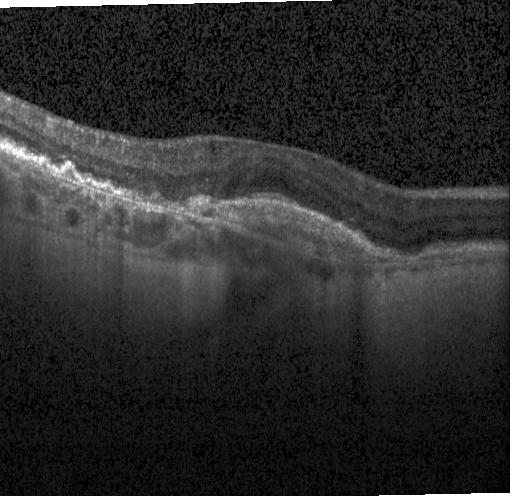
Macular OCT: choroidal neovascularization.